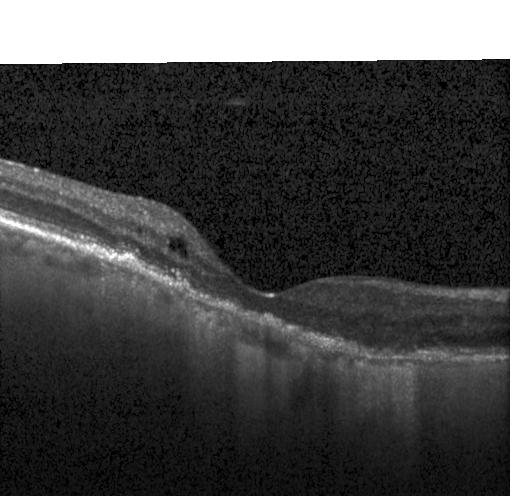 OCT line scan
CNV.